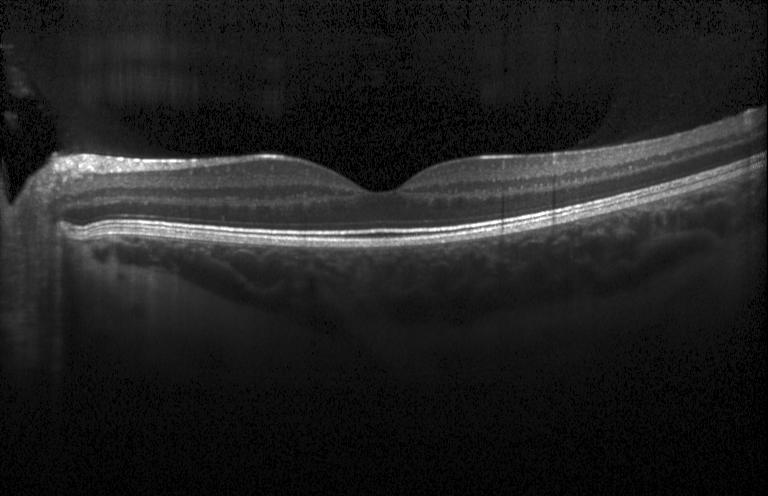
The scan shows no choroidal neovascularization, no diabetic macular edema, and no drusen.